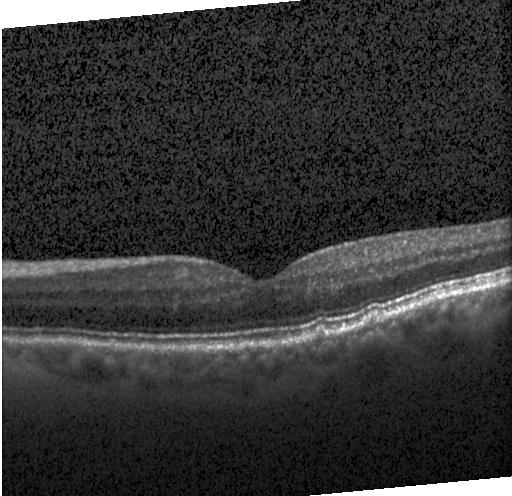

Heidelberg Spectralis. Spectral-domain OCT. Optical coherence tomography B-scan. Horizontal scan through the fovea — This B-scan demonstrates drusen.